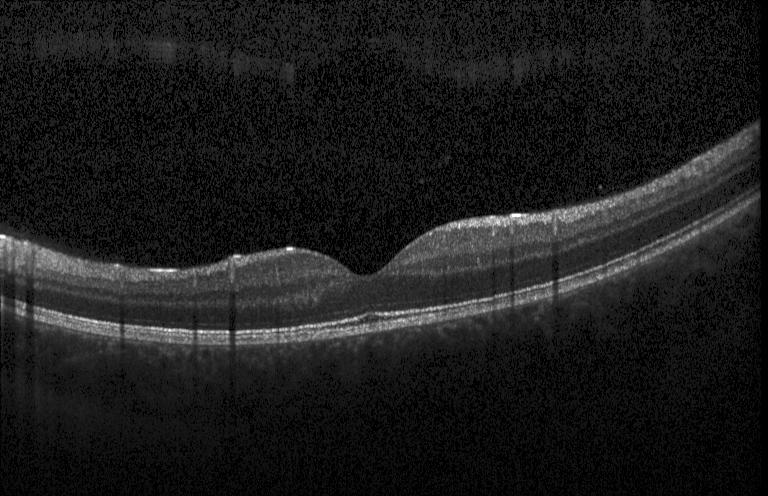
OCT B-scan. The scan shows no CNV, no DME, and no drusen.